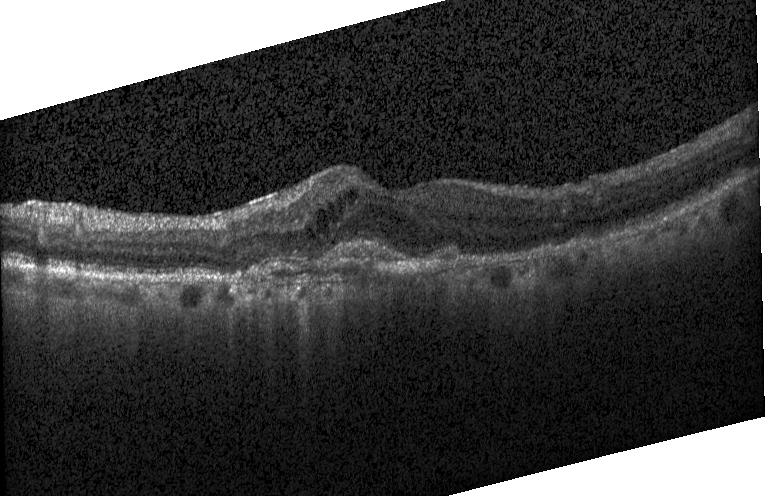

Acquired on a Heidelberg Spectralis, macular scan, optical coherence tomography scan, spectral-domain OCT. The scan shows CNV.